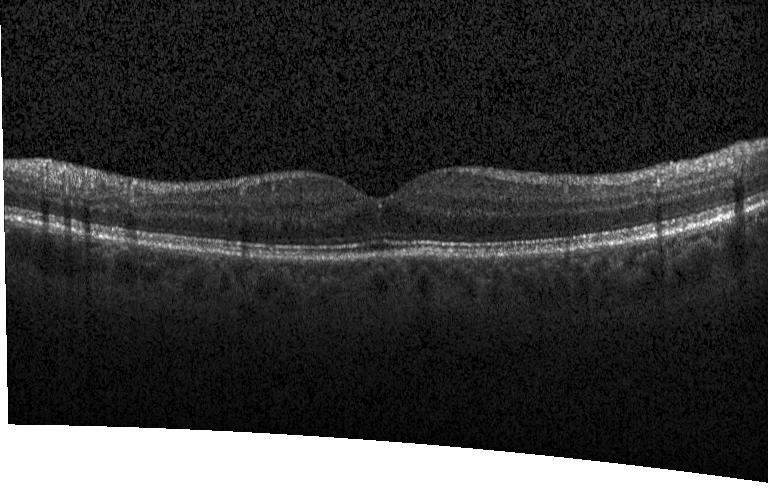 Macular scan · retinal OCT cross-section · spectral-domain OCT · acquired on a Heidelberg Spectralis
Finding: no CNV, no DME, and no drusen.